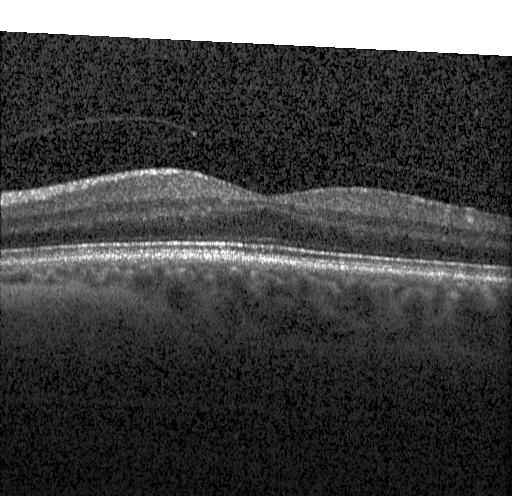

OCT line scan. Assessment: no evidence of choroidal neovascularization, diabetic macular edema, or drusen.